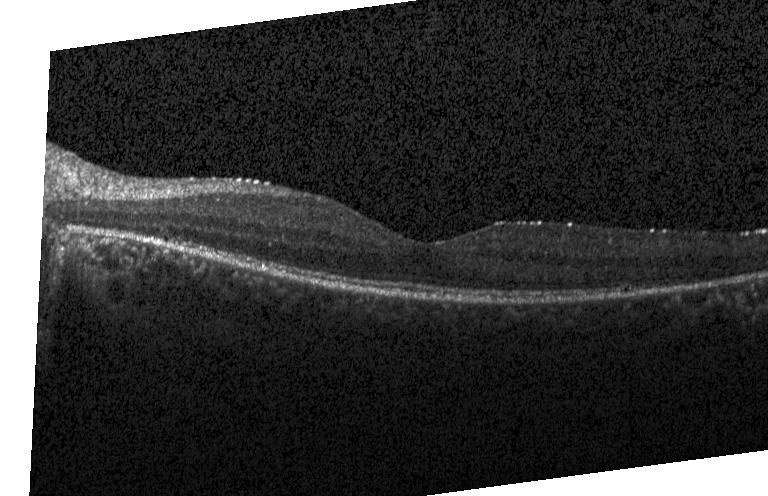

Macular OCT: no evidence of CNV, DME, or drusen.